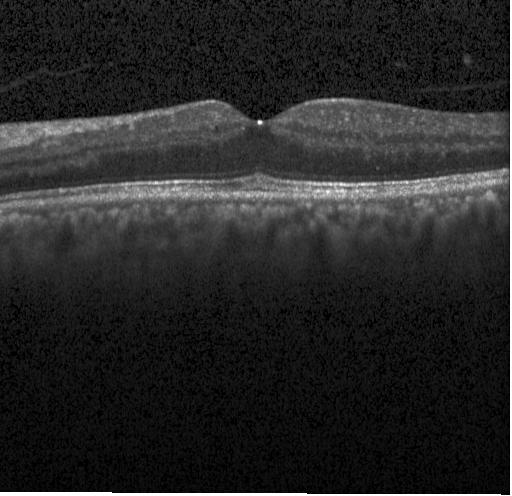
OCT line scan. Finding: no choroidal neovascularization, diabetic macular edema, or drusen.